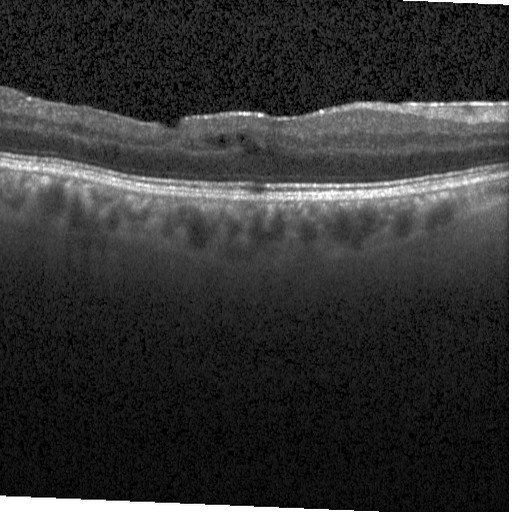 OCT line scan
Diagnosis: DME.